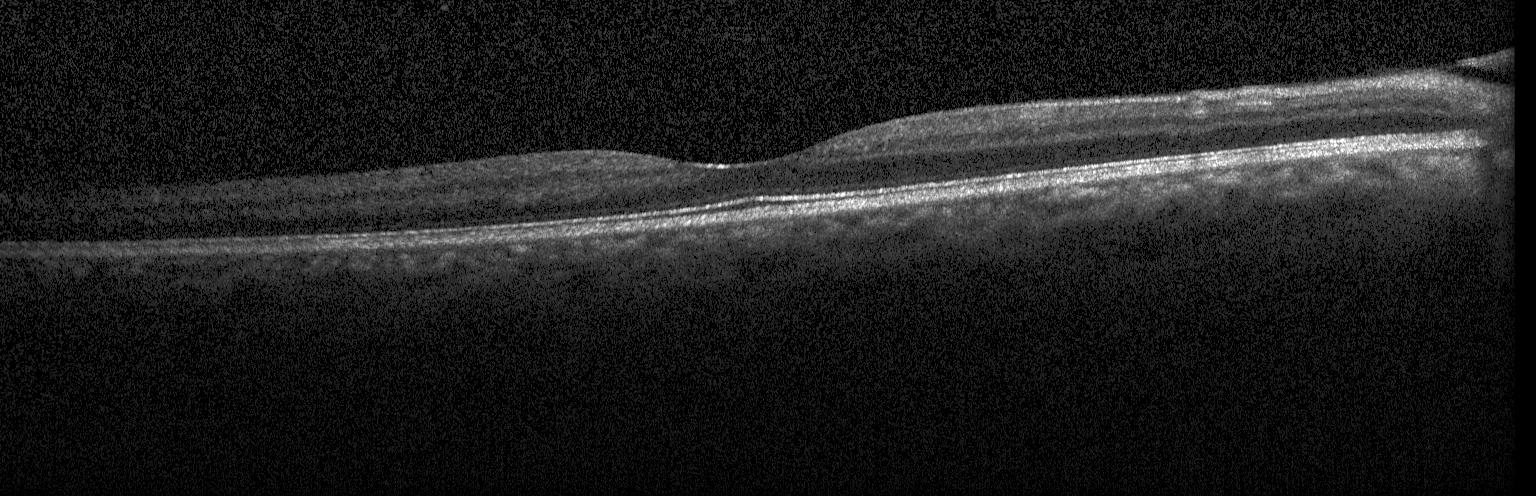
OCT B-scan. Horizontal scan through the fovea — OCT finding: no CNV, no DME, and no drusen.